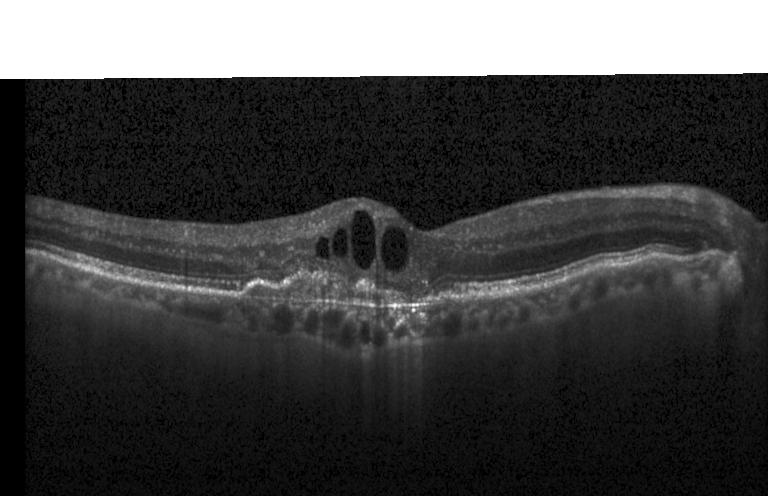 Acquired on a Heidelberg Spectralis · centered on the fovea · retinal OCT cross-section · SD-OCT — Diagnosis: a choroidal neovascular membrane.